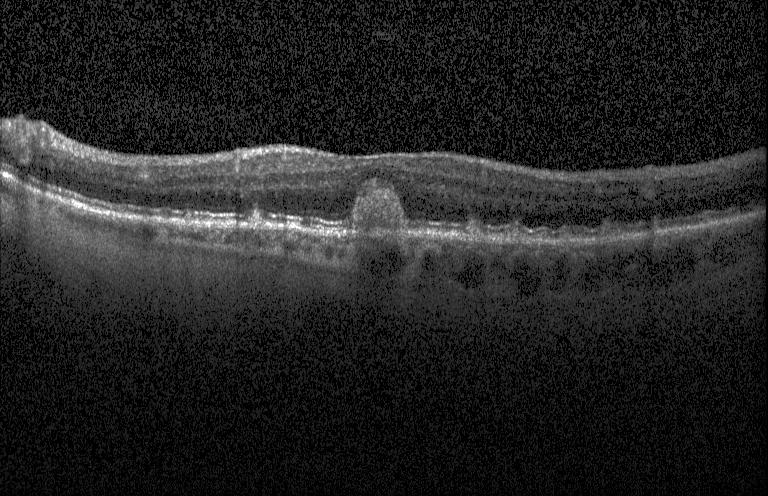 Centered on the fovea, acquired on a Heidelberg Spectralis, optical coherence tomography scan, spectral-domain OCT.
Dx: choroidal neovascularization.